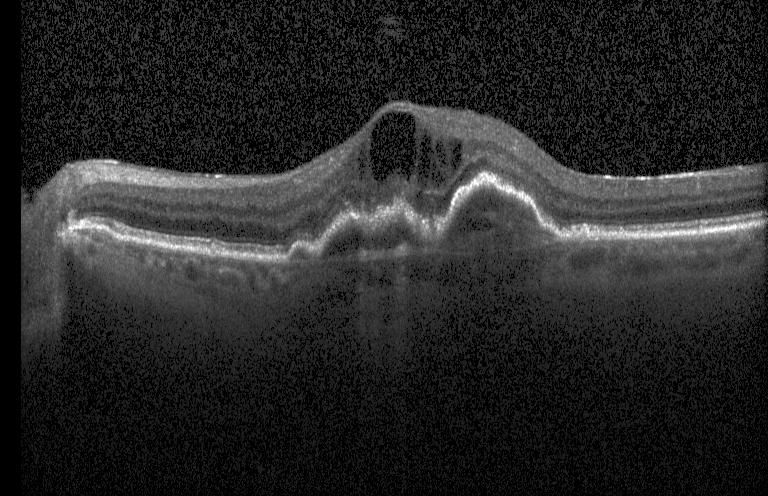
Retinal OCT B-scan · spectral-domain OCT
Assessment: a choroidal neovascular membrane.